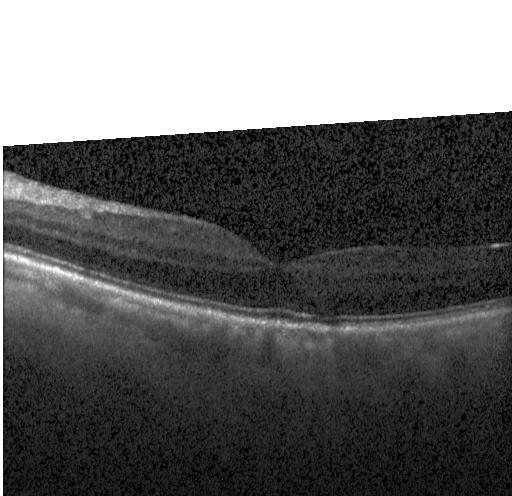 Impression: no choroidal neovascularization, diabetic macular edema, or drusen.